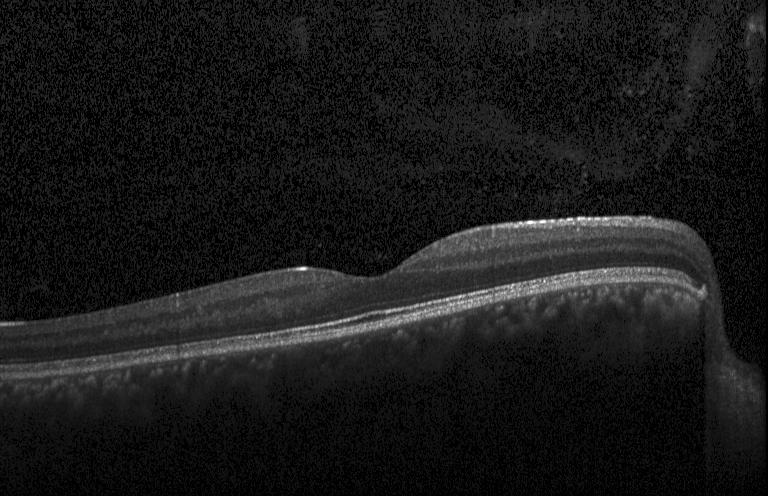
Spectral-domain OCT; optical coherence tomography scan; centered on the fovea.
The scan shows no evidence of choroidal neovascularization, diabetic macular edema, or drusen.